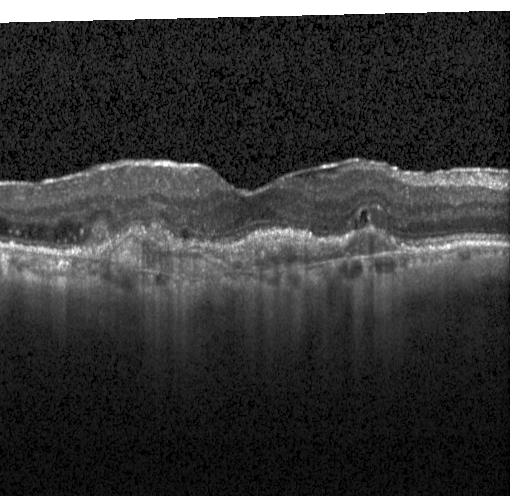

Retinal OCT cross-section
Diagnosis: CNV.